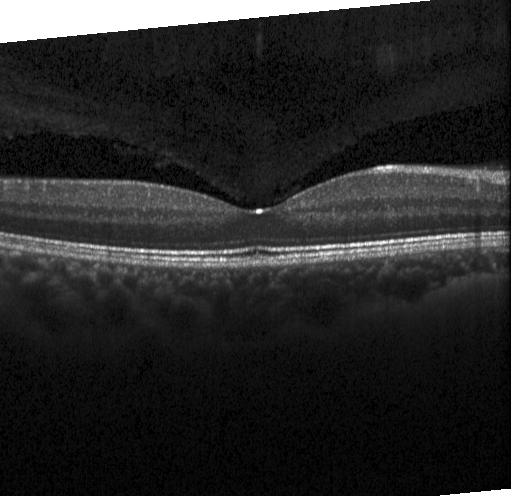
Macular scan, optical coherence tomography B-scan, SD-OCT, Heidelberg Spectralis OCT system. Diagnosis: no choroidal neovascularization, no diabetic macular edema, and no drusen.